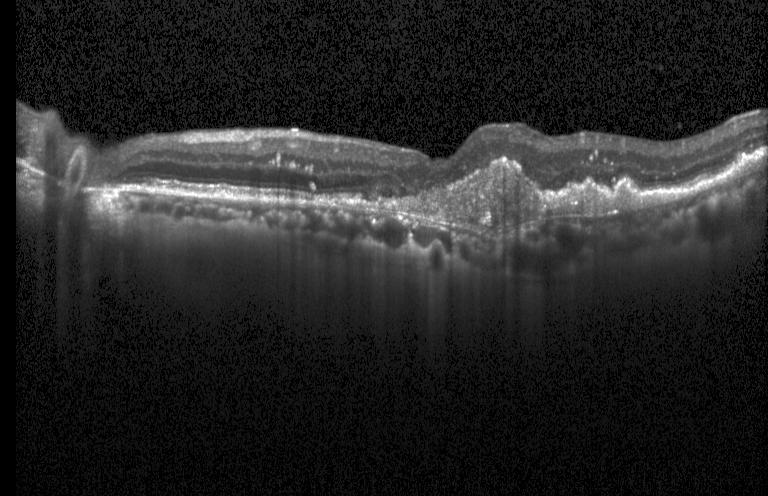
Acquired on a Heidelberg Spectralis · retinal OCT cross-section · macular scan · SD-OCT — Diagnosis: a choroidal neovascular membrane.